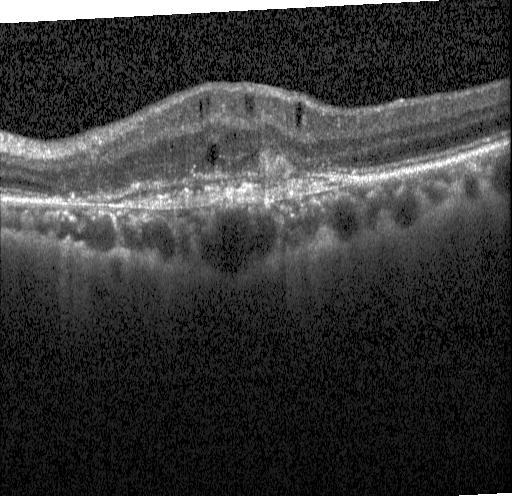

Acquired on a Heidelberg Spectralis, SD-OCT, OCT line scan. Diagnosis: choroidal neovascularization.